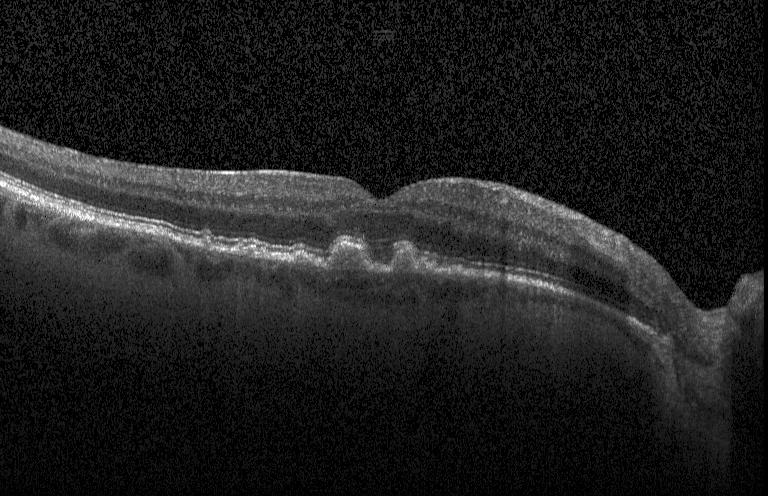 Spectral-domain OCT, retinal OCT cross-section.
Finding: multiple drusen.